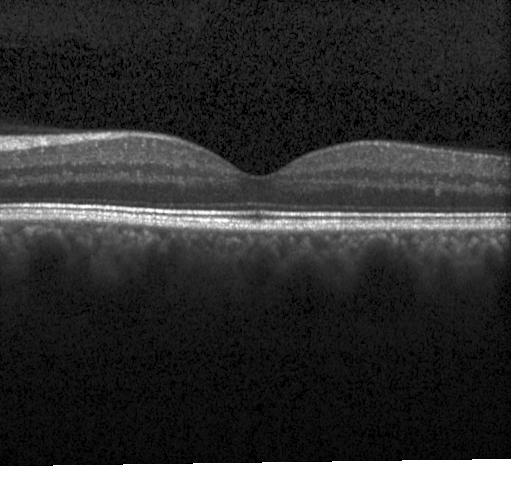

OCT line scan.
Assessment: no choroidal neovascularization, no diabetic macular edema, and no drusen.